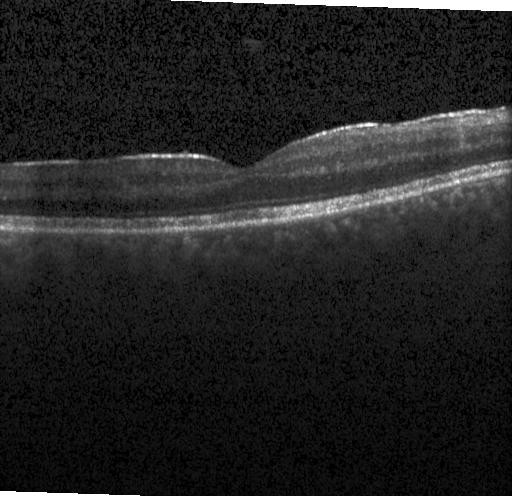 Optical coherence tomography scan. No CNV, DME, or drusen.